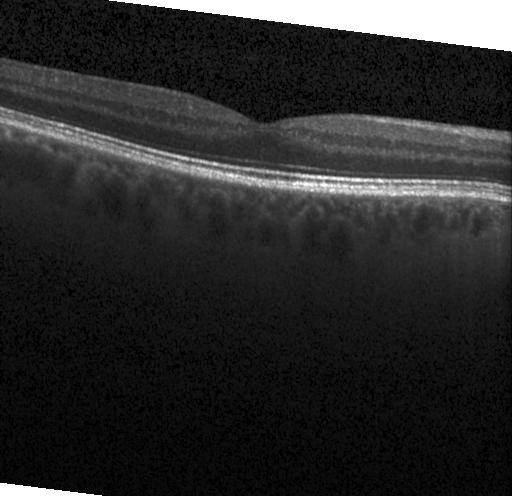
OCT B-scan showing no choroidal neovascularization, diabetic macular edema, or drusen.